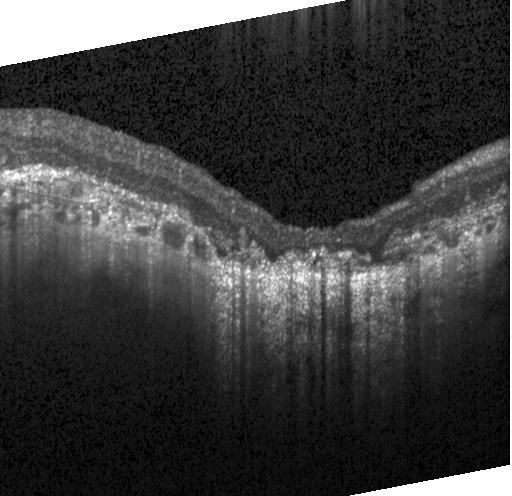

Impression: a choroidal neovascular membrane.